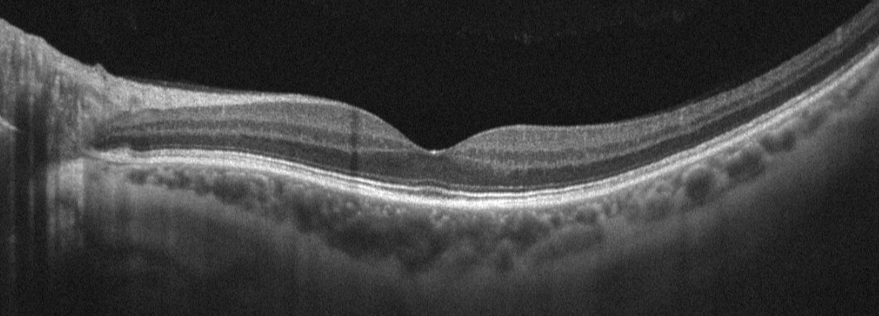
Impression: no evidence of AMD, DME, ERM, RAO, RVO, or VID.